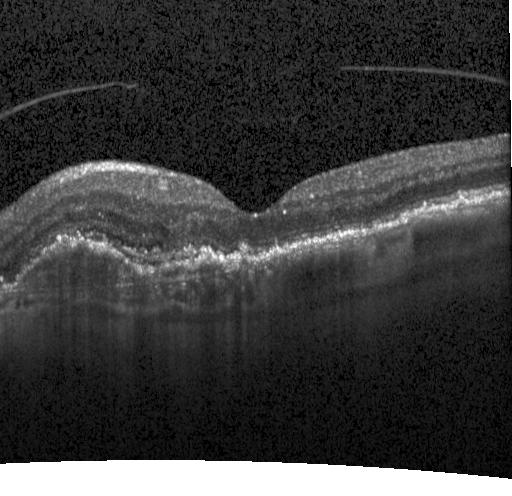 Retinal OCT B-scan; acquired on a Heidelberg Spectralis; spectral-domain optical coherence tomography; through the macula. A choroidal neovascular membrane.